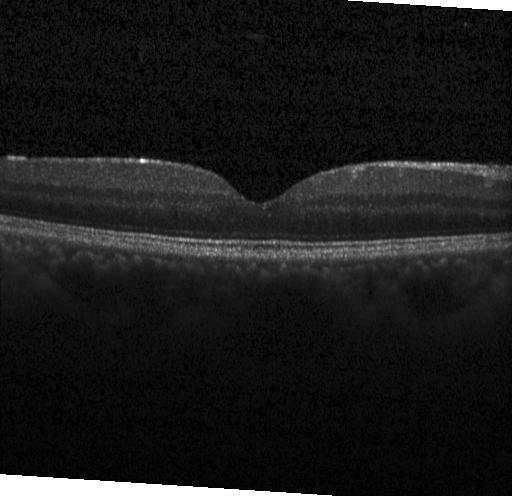 Spectral-domain OCT, instrument: Heidelberg Spectralis, OCT line scan, fovea-centered.
Dx: no evidence of choroidal neovascularization, diabetic macular edema, or drusen.